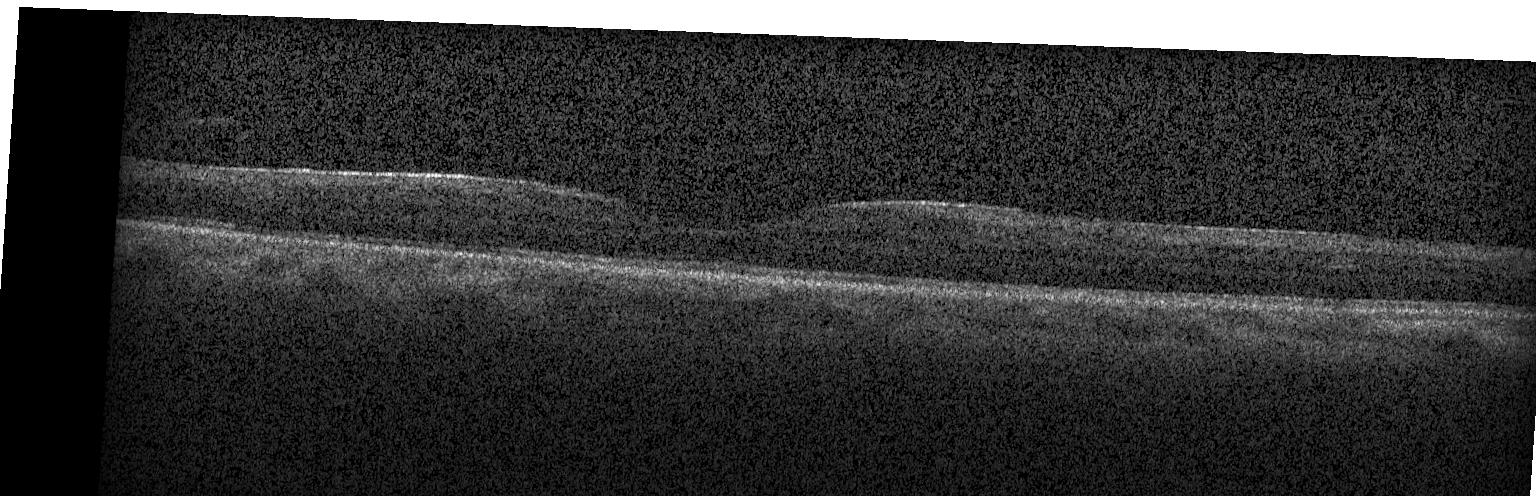

Heidelberg Spectralis OCT system; OCT line scan; spectral-domain OCT; through the macula. This B-scan demonstrates neither choroidal neovascularization, diabetic macular edema, nor drusen.